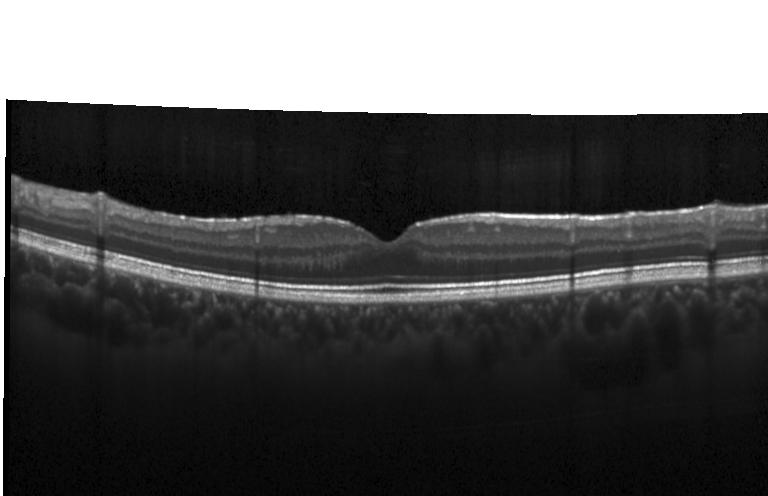

OCT finding: no evidence of CNV, DME, or drusen.